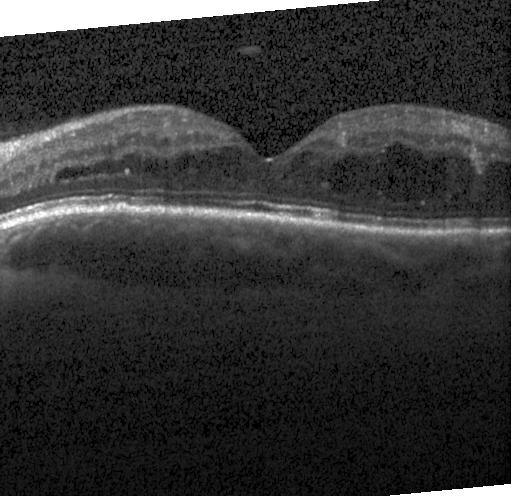 Macular OCT: diabetic macular edema.